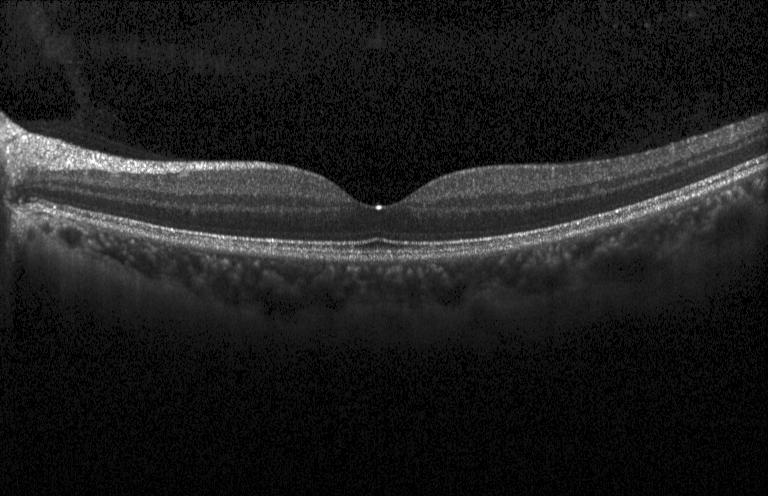 Dx: no CNV, DME, or drusen.